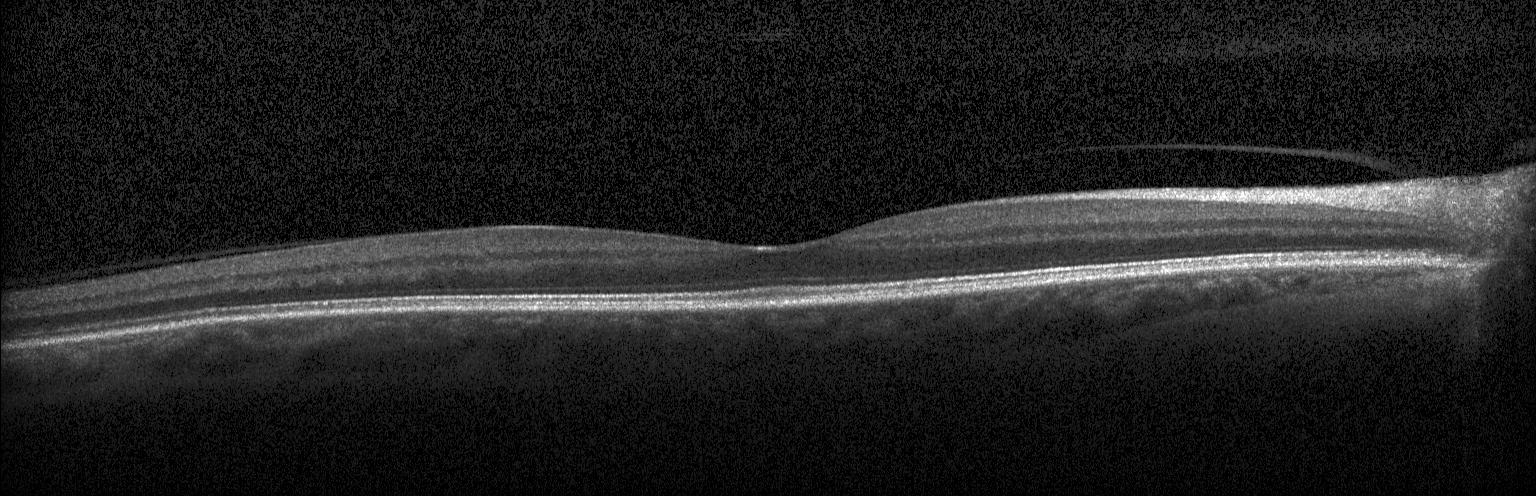

Optical coherence tomography B-scan. Instrument: Heidelberg Spectralis. Horizontal scan through the fovea. SD-OCT. Finding: no evidence of choroidal neovascularization, diabetic macular edema, or drusen.